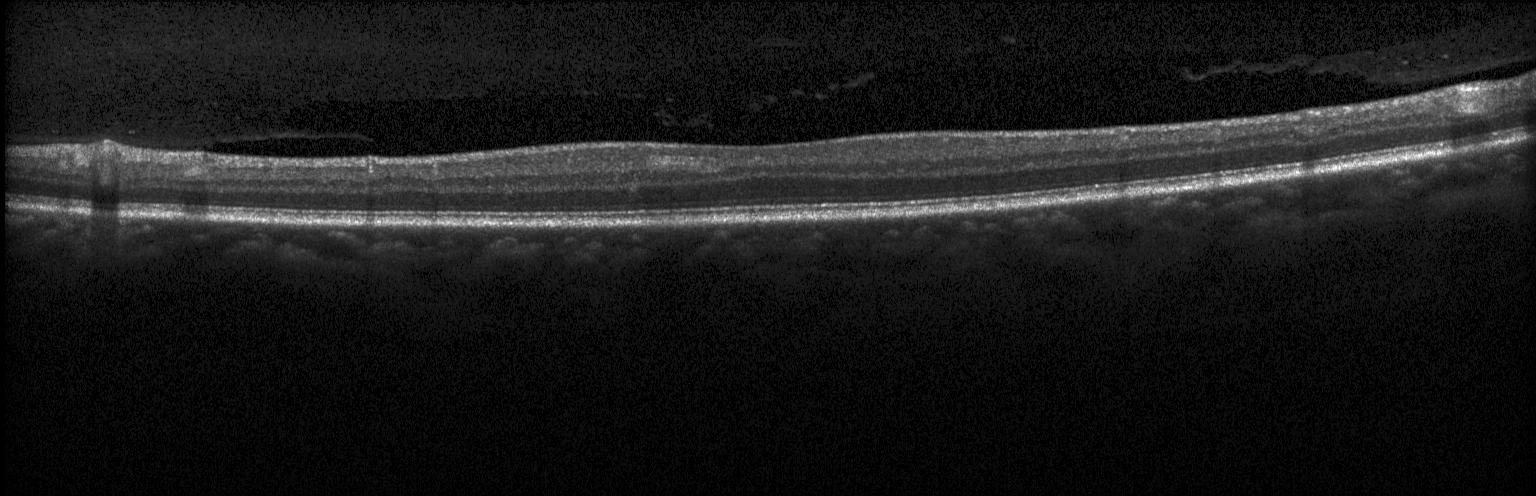 OCT line scan, through the macula. This B-scan demonstrates no choroidal neovascularization, diabetic macular edema, or drusen.